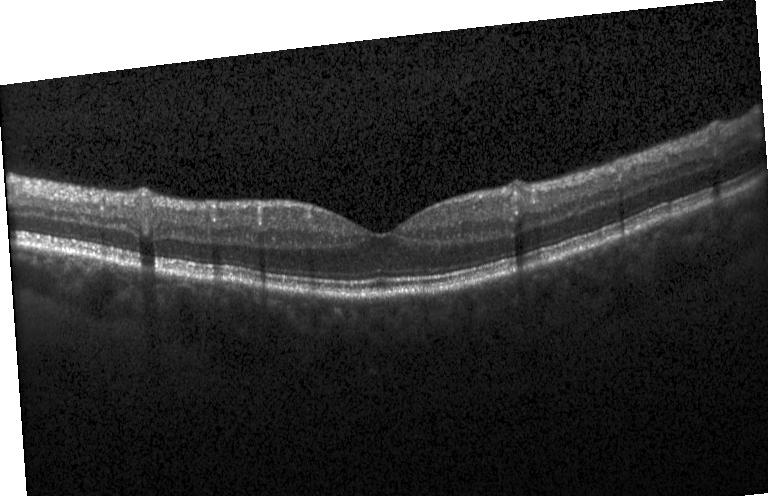

Macular scan. Instrument: Heidelberg Spectralis. Retinal OCT B-scan. Spectral-domain OCT — Assessment: no choroidal neovascularization, no diabetic macular edema, and no drusen.